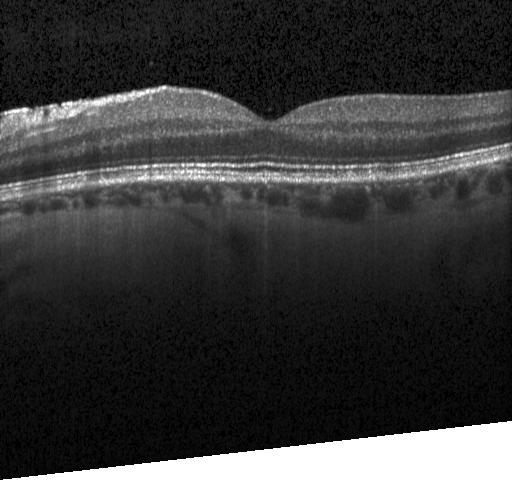
Spectral-domain OCT, macular scan, instrument: Heidelberg Spectralis, retinal OCT cross-section — Assessment: no CNV, no DME, and no drusen.